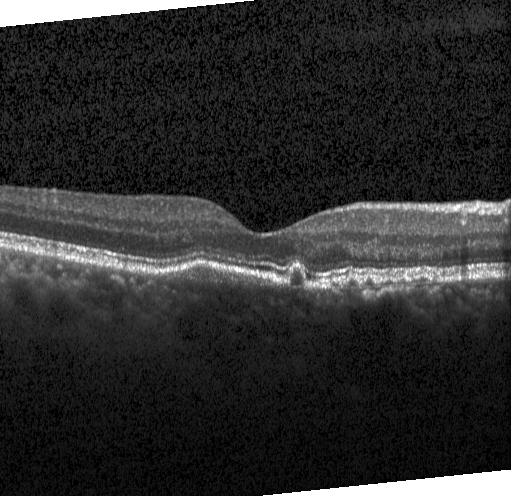 Spectral-domain optical coherence tomography. OCT B-scan.
Diagnosis: multiple drusen.